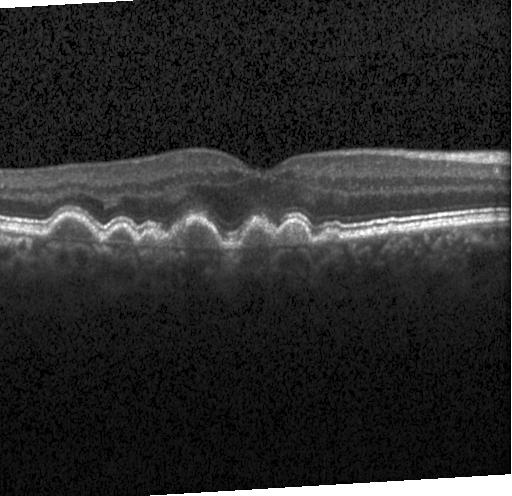
Retinal OCT cross-section.
Impression: multiple drusen.